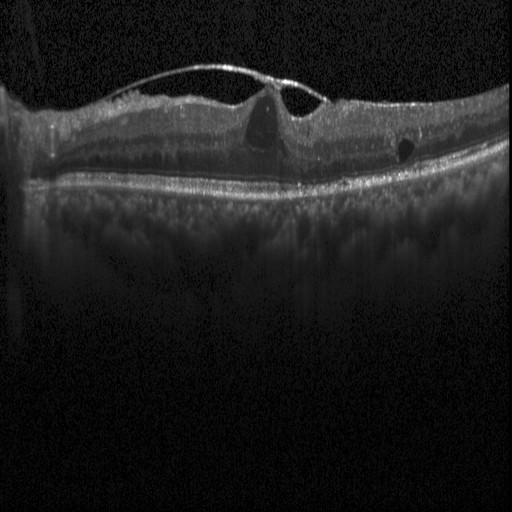 Macular OCT: DME.